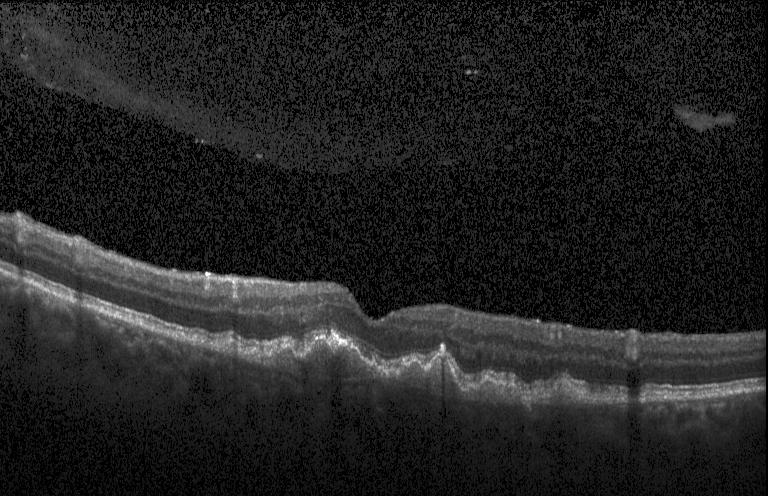

Macular scan; optical coherence tomography B-scan
This B-scan demonstrates a choroidal neovascular membrane.